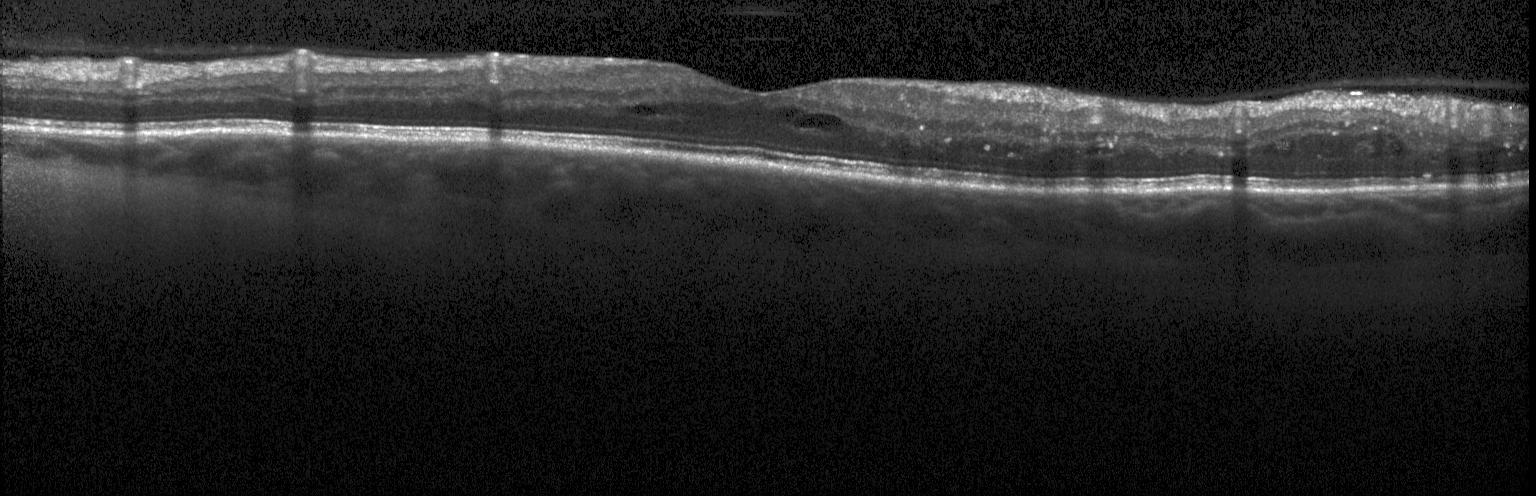 Impression: diabetic macular edema.